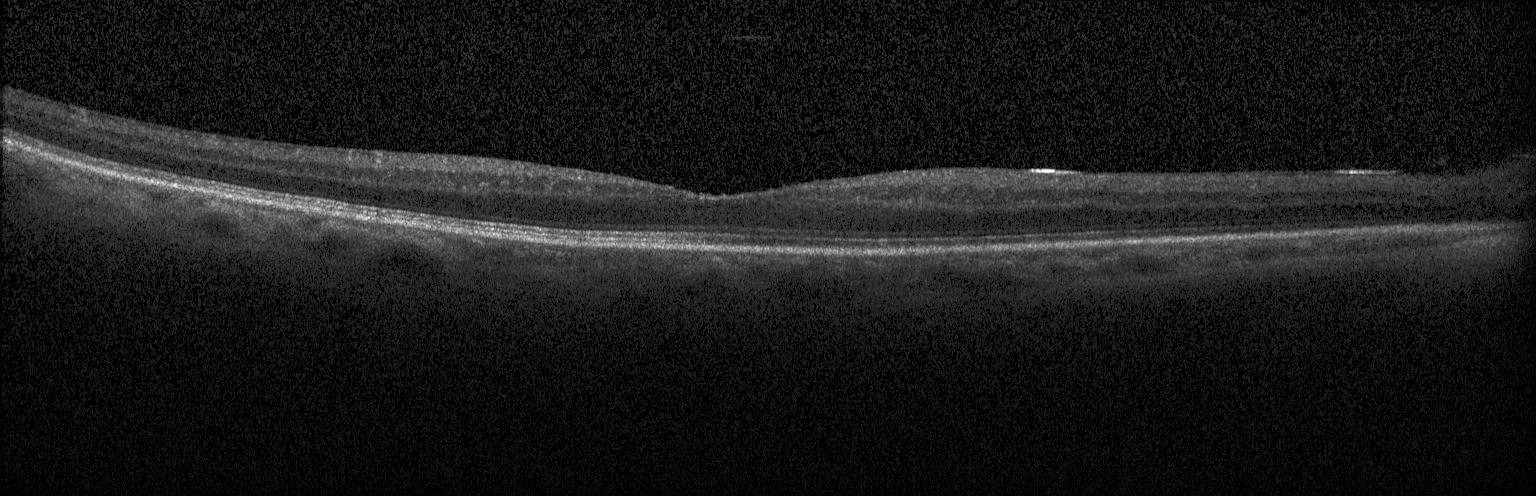
Spectral-domain optical coherence tomography. Heidelberg Spectralis OCT system. Retinal OCT cross-section. Horizontal scan through the fovea.
Finding: no evidence of CNV, DME, or drusen.